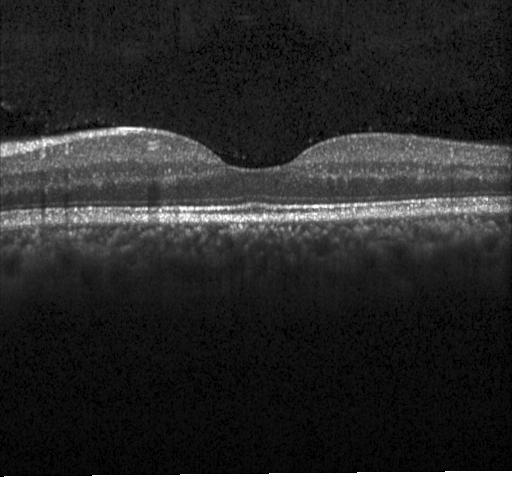
Diagnosis: neither choroidal neovascularization, diabetic macular edema, nor drusen.